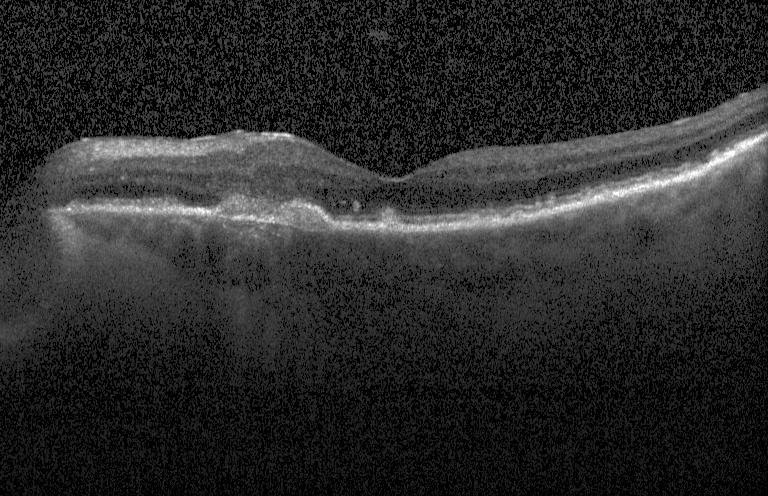

Retinal OCT B-scan.
Diagnosis: choroidal neovascularization.